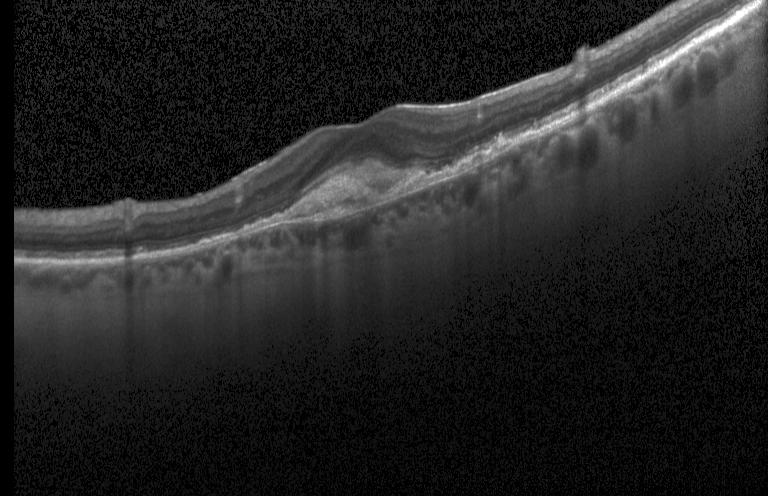 Macular OCT demonstrating choroidal neovascularization (CNV).